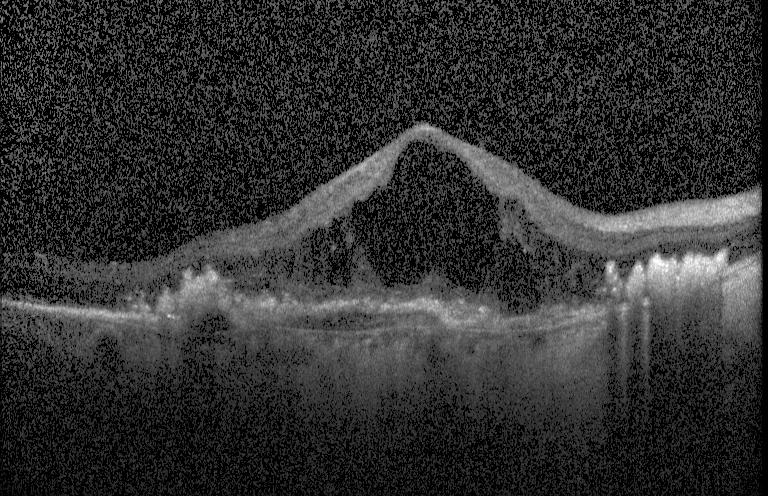

Horizontal scan through the fovea; OCT line scan. Impression: a choroidal neovascular membrane.